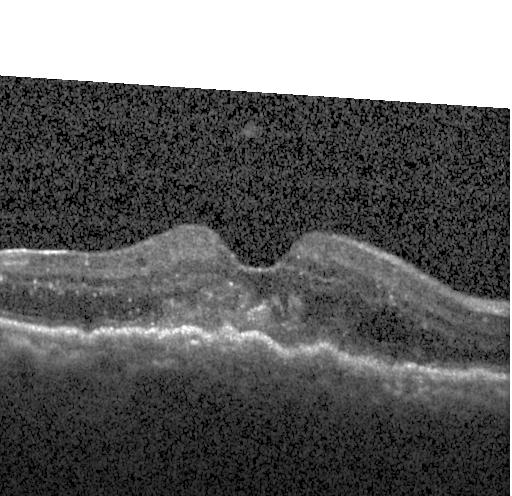
OCT scan showing a choroidal neovascular membrane.